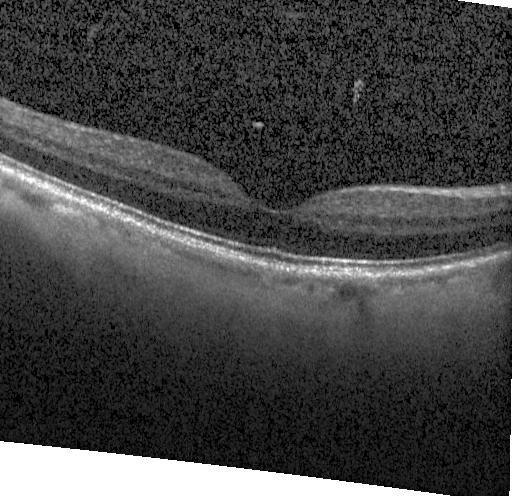 Retinal OCT B-scan. Macular OCT: neither choroidal neovascularization, diabetic macular edema, nor drusen.